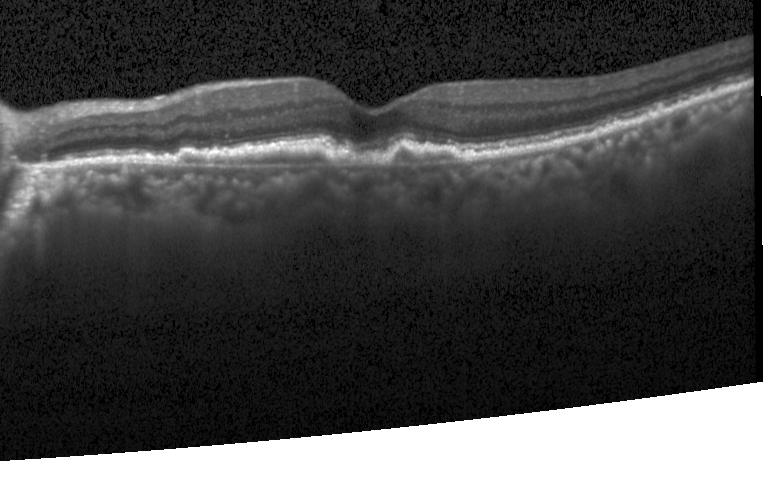 Spectral-domain OCT; retinal OCT cross-section; horizontal scan through the fovea.
This B-scan demonstrates a choroidal neovascular membrane.